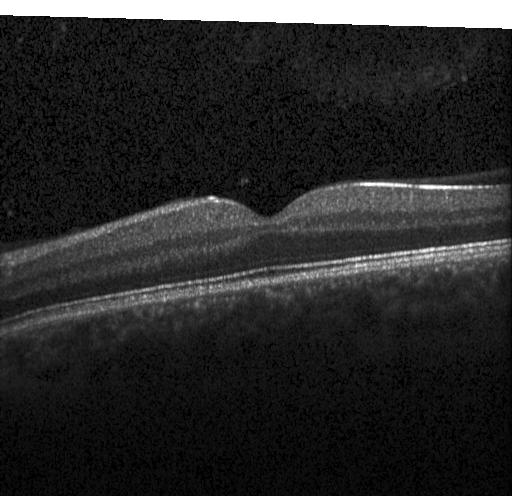 No choroidal neovascularization, diabetic macular edema, or drusen.